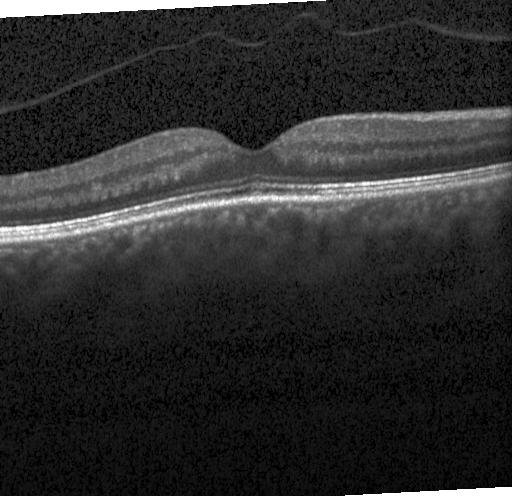 Retinal OCT B-scan — Finding: no CNV, no DME, and no drusen.